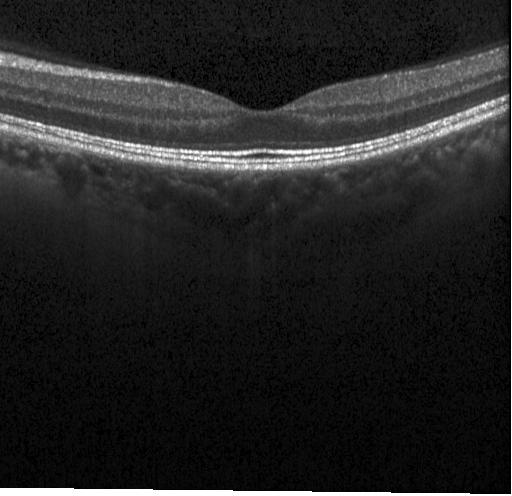 OCT line scan; spectral-domain optical coherence tomography; Heidelberg Spectralis OCT system; horizontal scan through the fovea — Macular OCT: no choroidal neovascularization, no diabetic macular edema, and no drusen.